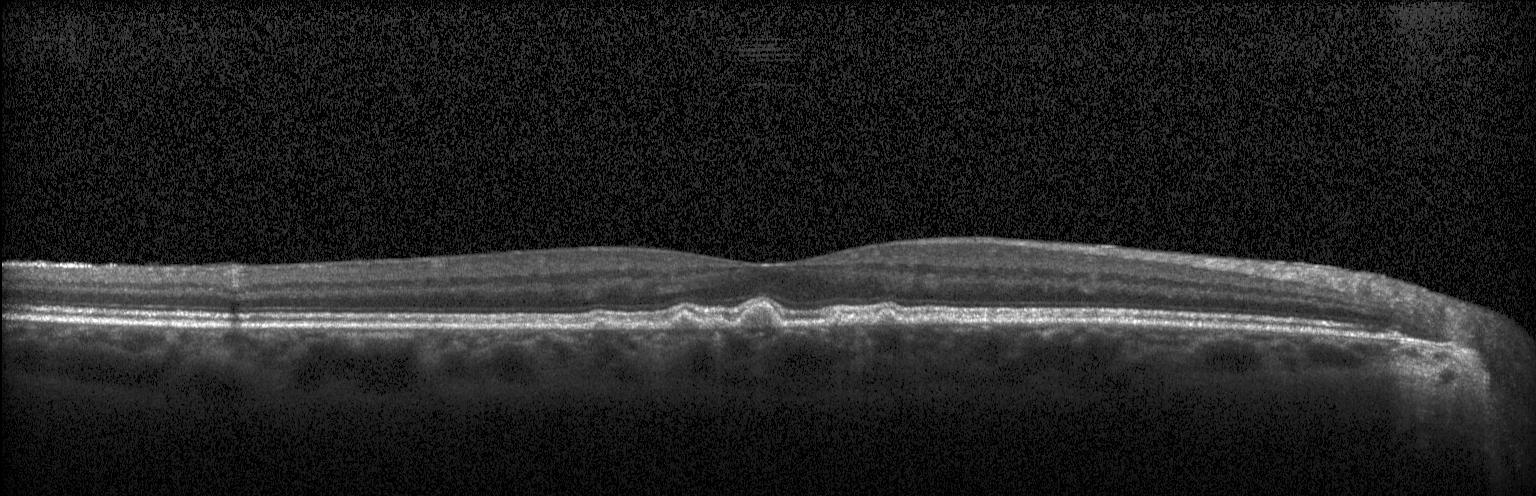
Heidelberg Spectralis OCT system · through the macula · optical coherence tomography B-scan — Impression: sub-RPE drusenoid deposits.